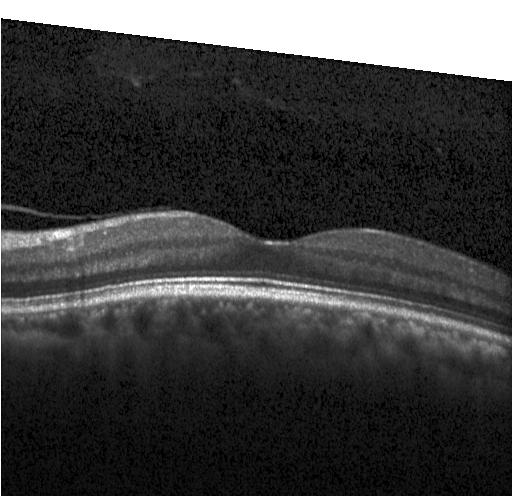
Impression: no evidence of choroidal neovascularization, diabetic macular edema, or drusen.